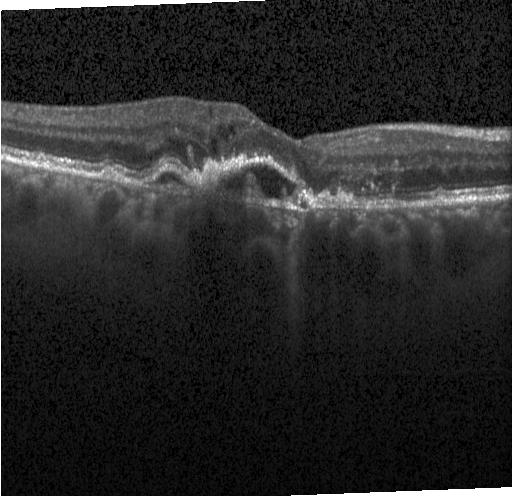

Diagnosis: choroidal neovascularization (CNV).